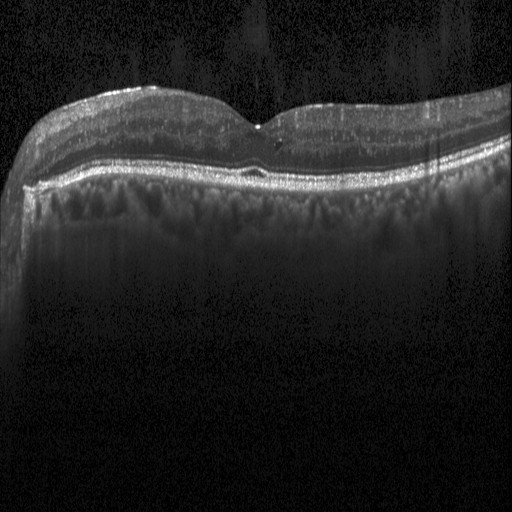
SD-OCT, fovea-centered, optical coherence tomography scan.
The scan shows diabetic macular edema.